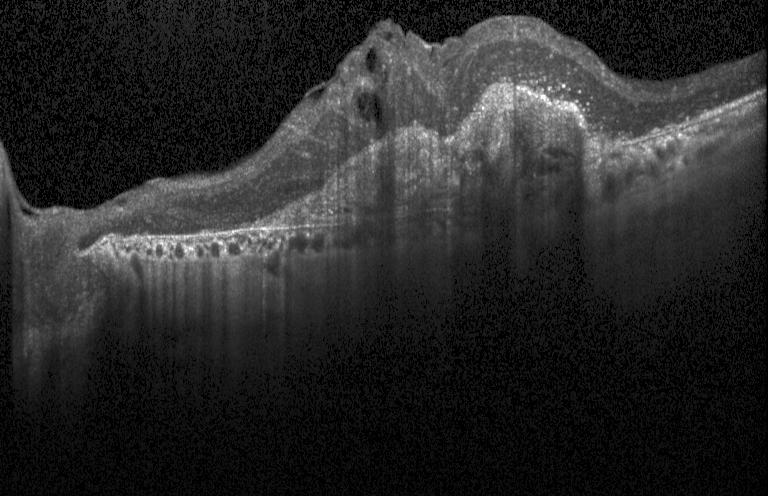
Optical coherence tomography scan; instrument: Heidelberg Spectralis; spectral-domain OCT — Impression: a choroidal neovascular membrane.